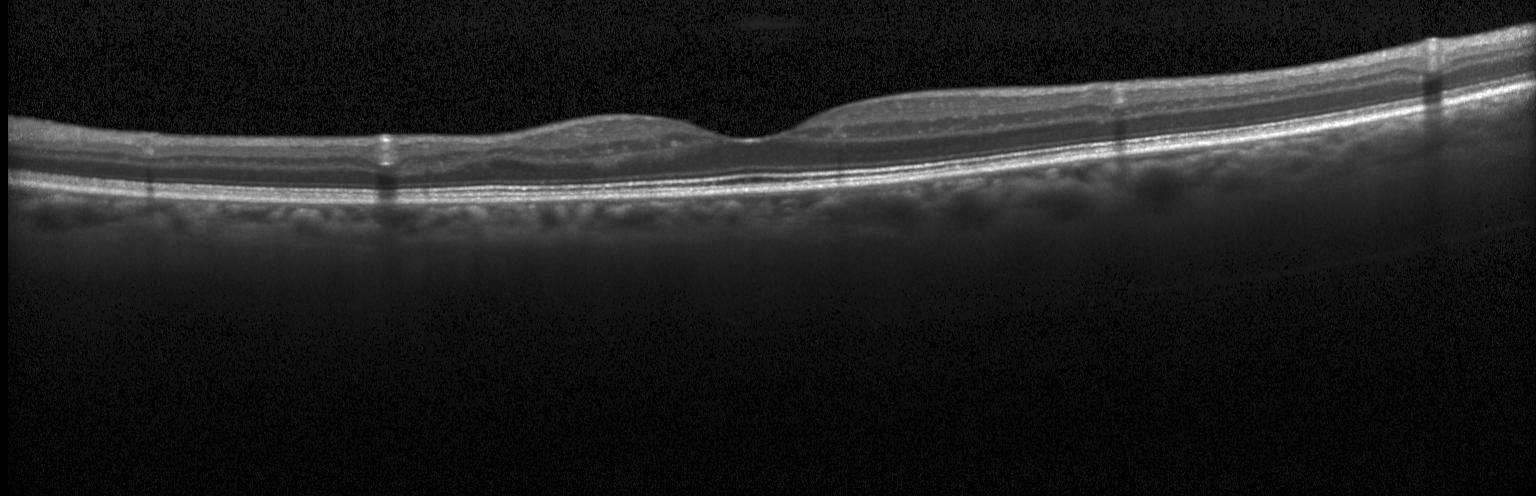

Retinal OCT cross-section.
The scan shows no evidence of choroidal neovascularization, diabetic macular edema, or drusen.